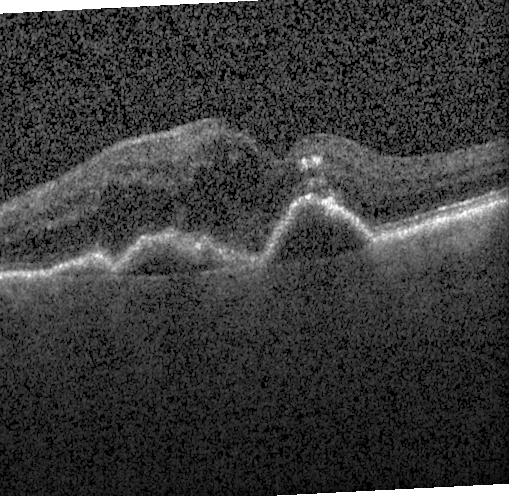
Spectral-domain OCT · horizontal scan through the fovea · optical coherence tomography scan · Heidelberg Spectralis.
Impression: a choroidal neovascular membrane.